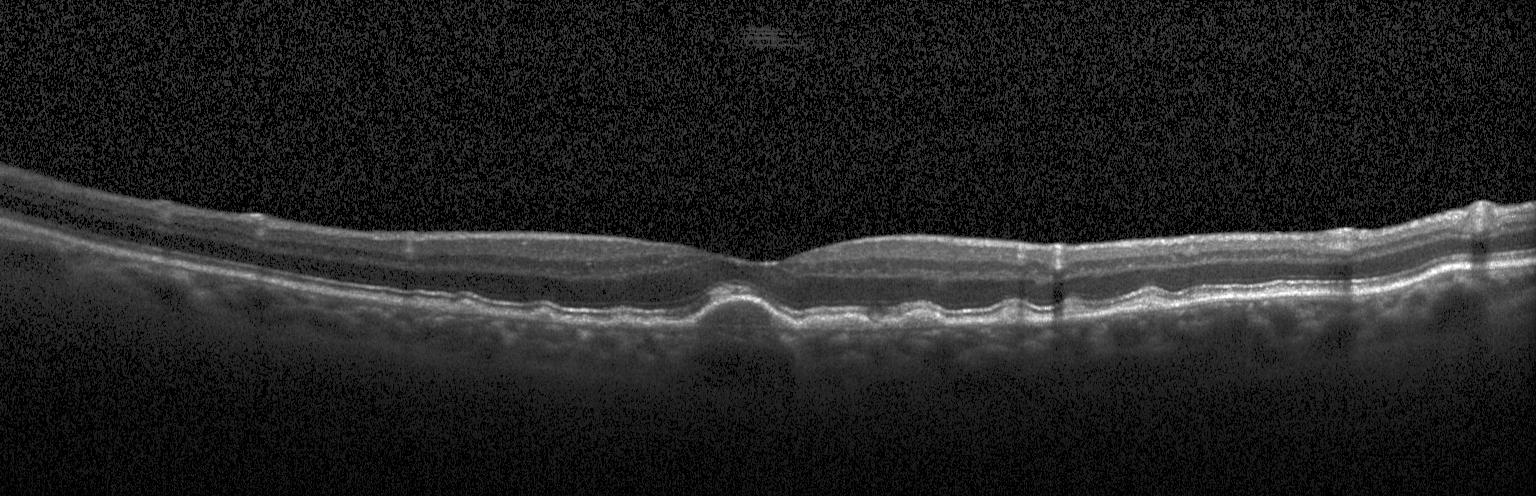

Diagnosis: drusen.